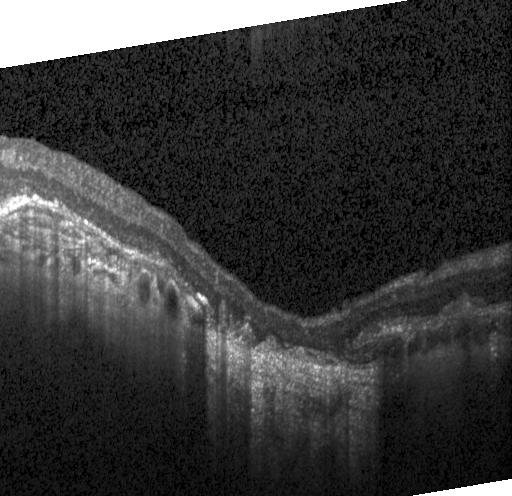 Heidelberg Spectralis OCT system; OCT B-scan; horizontal scan through the fovea.
OCT finding: a choroidal neovascular membrane.